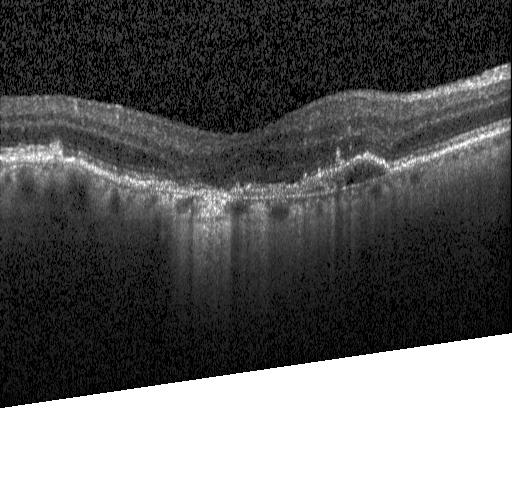

The scan shows choroidal neovascularization (CNV).